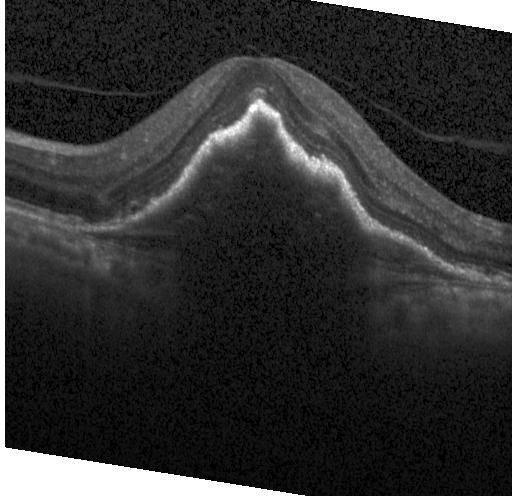

Spectral-domain optical coherence tomography. OCT B-scan — Assessment: choroidal neovascularization (CNV).